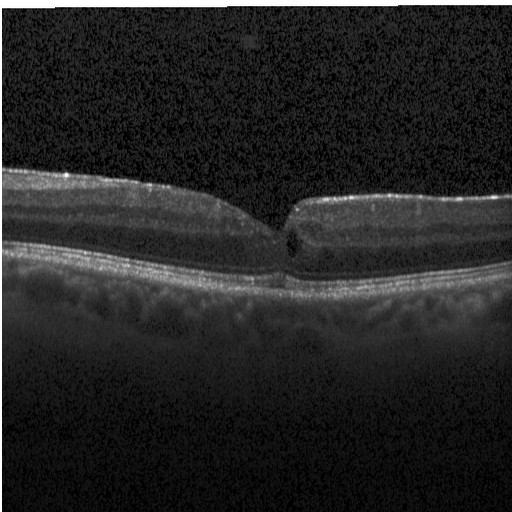

Finding: diabetic macular edema (DME).